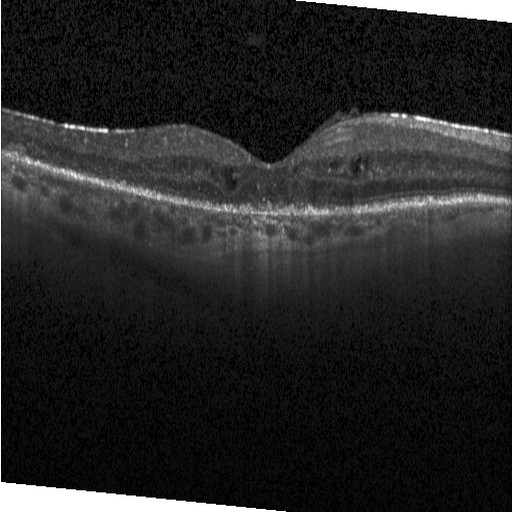 Spectral-domain optical coherence tomography; OCT B-scan; macular scan; instrument: Heidelberg Spectralis. Macular OCT: diabetic macular edema.